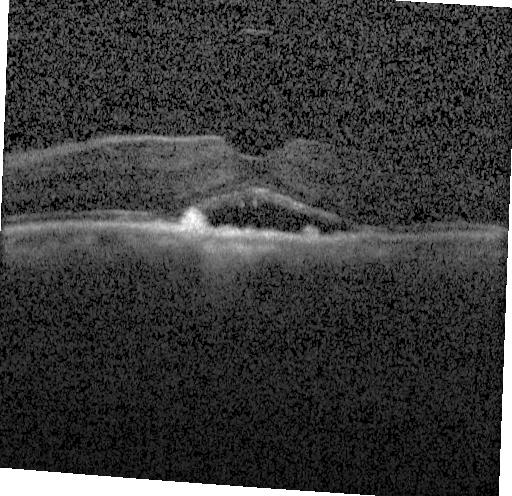 The scan shows CNV.